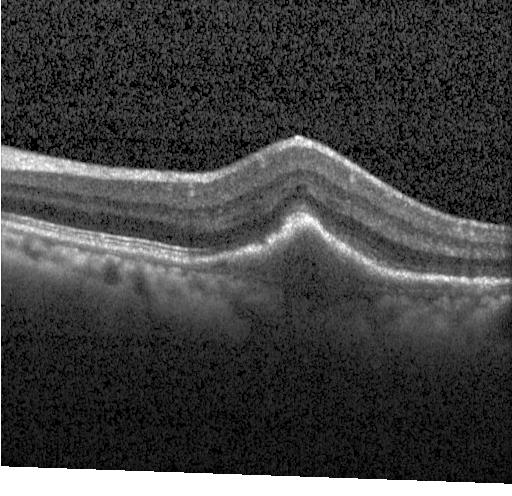

Assessment: choroidal neovascularization.